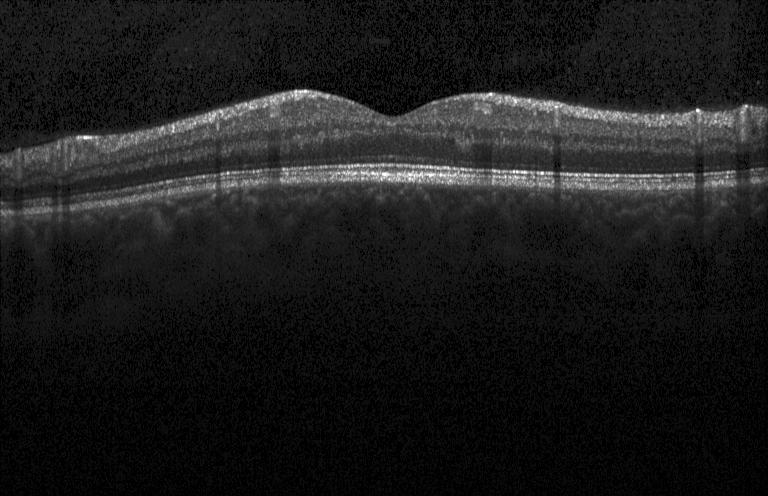
Retinal OCT cross-section.
Diagnosis: neither choroidal neovascularization, diabetic macular edema, nor drusen.